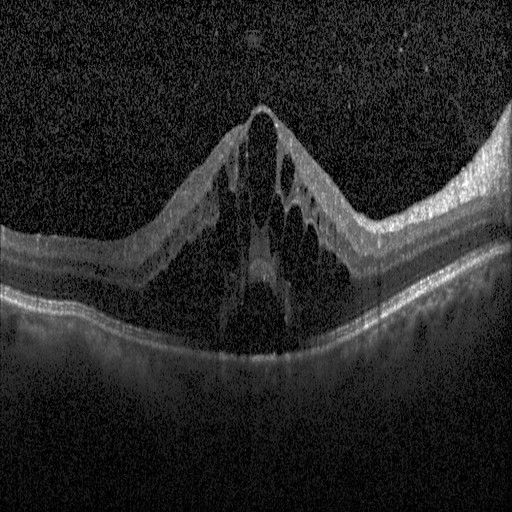 OCT finding: diabetic macular edema.